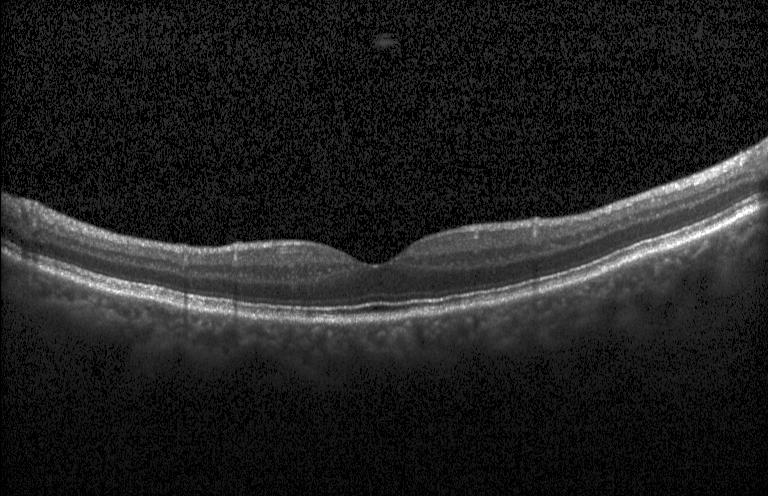 OCT B-scan
Diagnosis: no choroidal neovascularization, no diabetic macular edema, and no drusen.